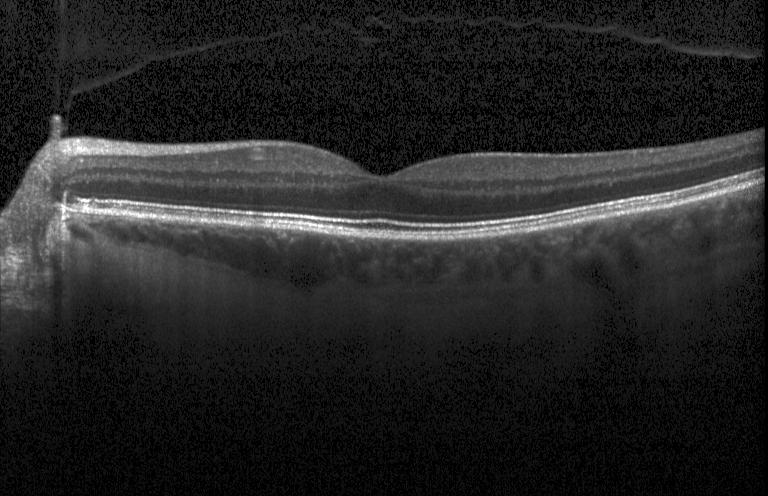 Macular OCT: no evidence of choroidal neovascularization, diabetic macular edema, or drusen.